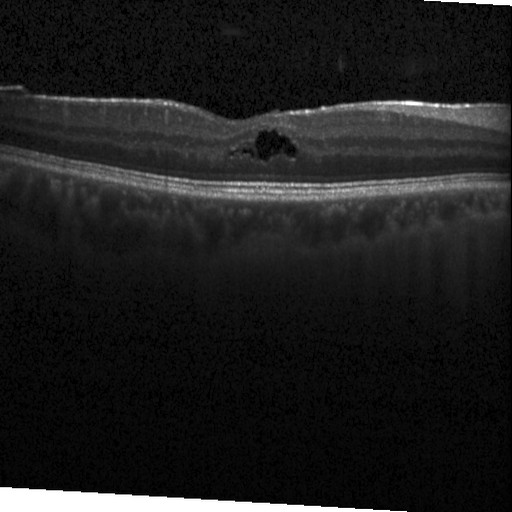 Retinal OCT B-scan.
Diagnosis: diabetic macular edema.